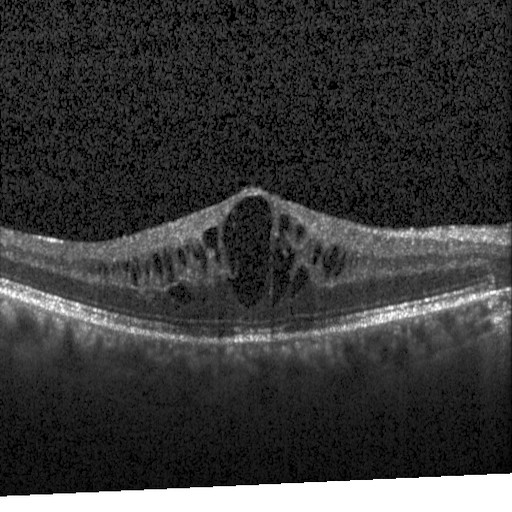 Dx: DME.